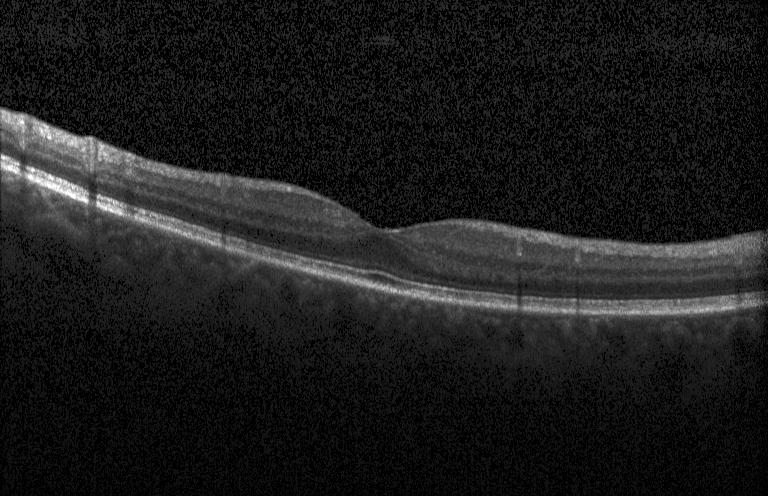 OCT line scan, spectral-domain OCT, instrument: Heidelberg Spectralis, through the macula. Impression: neither choroidal neovascularization, diabetic macular edema, nor drusen.